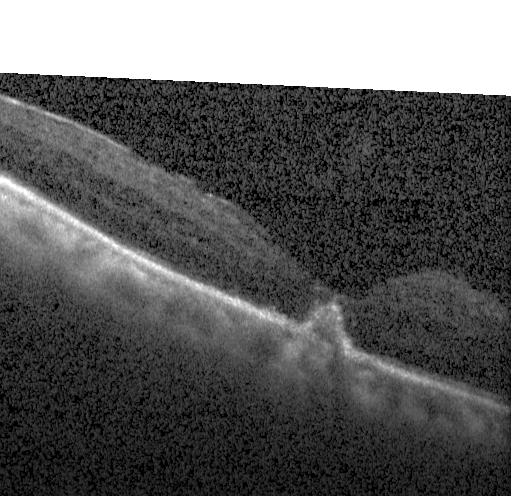
Finding: a choroidal neovascular membrane.